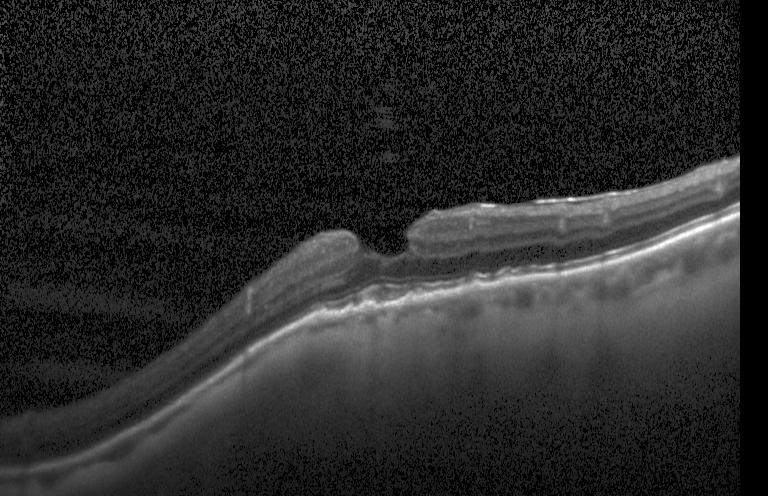

Retinal OCT cross-section showing drusen.